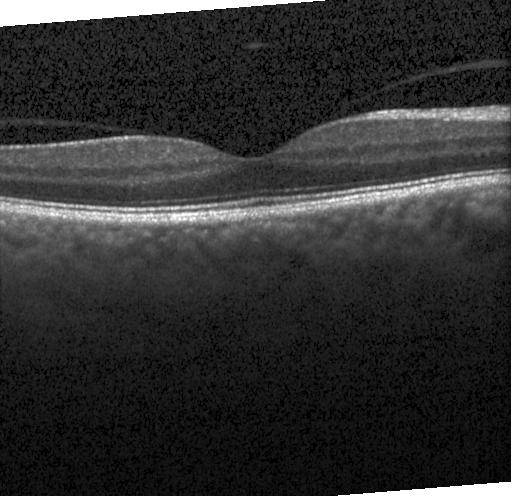

This B-scan demonstrates no choroidal neovascularization, diabetic macular edema, or drusen.